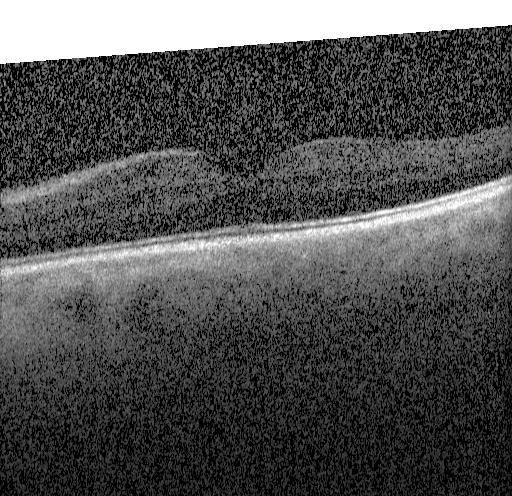
Macular OCT demonstrating neither choroidal neovascularization, diabetic macular edema, nor drusen.